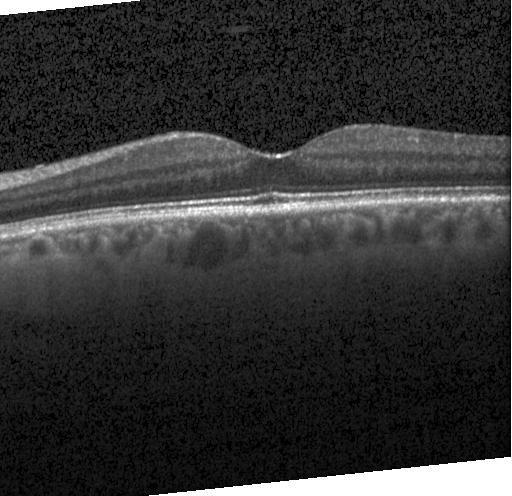

Spectral-domain OCT B-scan: no evidence of choroidal neovascularization, diabetic macular edema, or drusen.